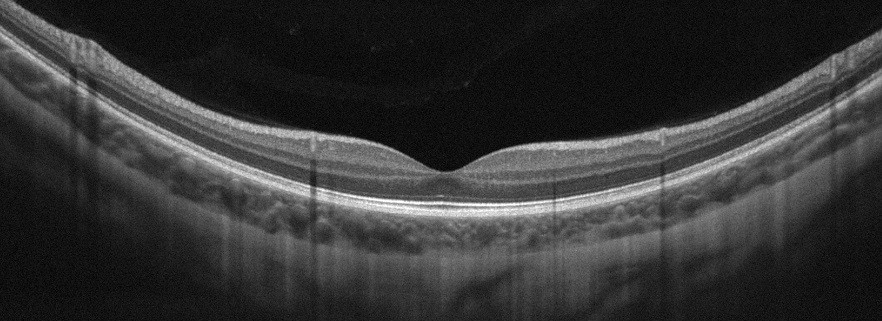 OCT B-scan, instrument: Optovue Avanti RTVue XR, fovea-centered. Impression: no evidence of AMD, DME, ERM, RAO, RVO, or VID.